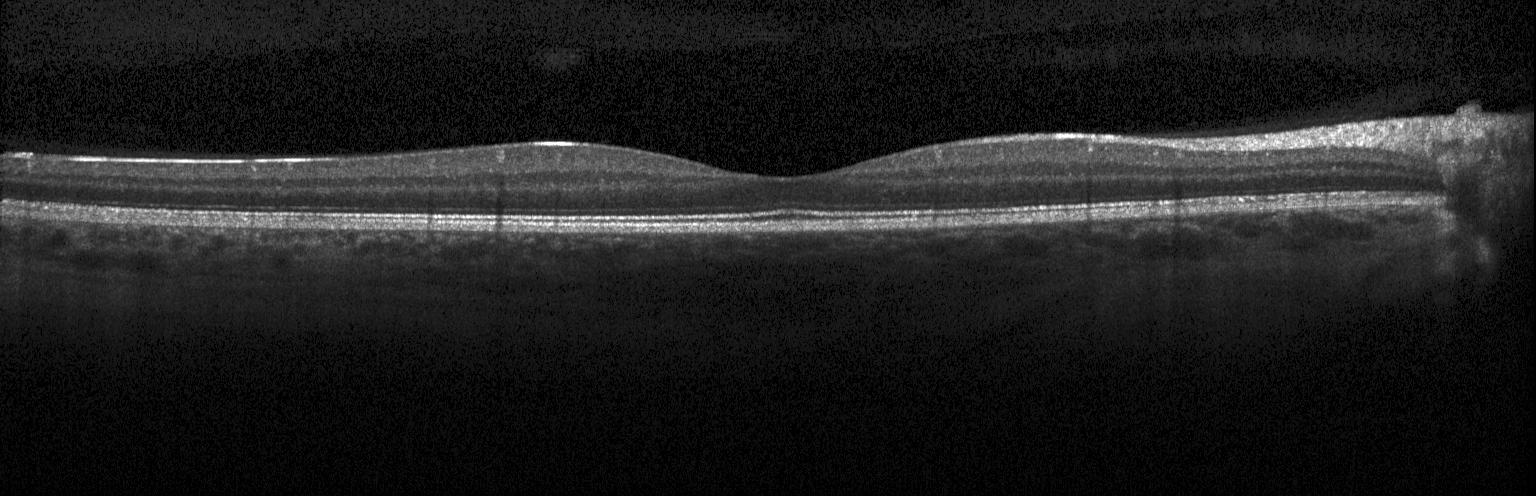
Retinal OCT B-scan. Impression: neither choroidal neovascularization, diabetic macular edema, nor drusen.